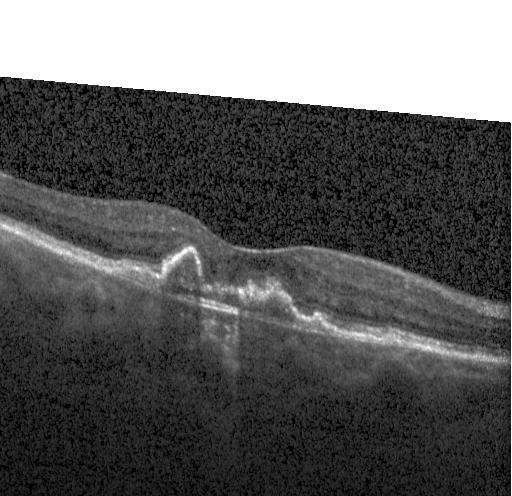
Acquired on a Heidelberg Spectralis · optical coherence tomography scan
Diagnosis: a choroidal neovascular membrane.